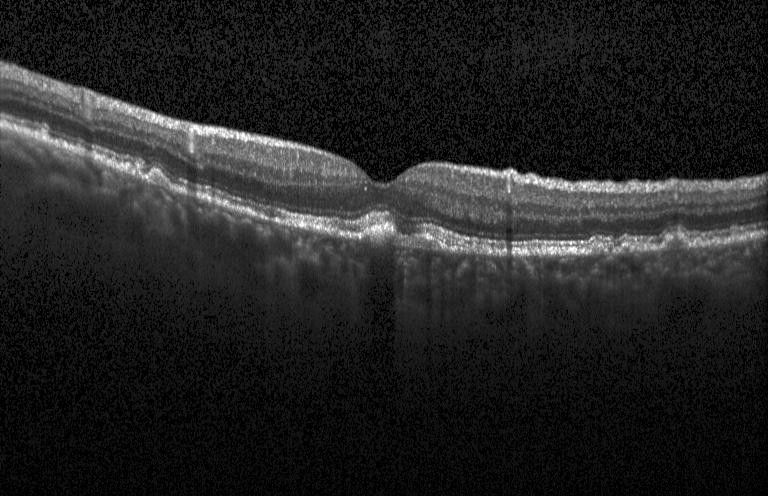

The scan shows sub-RPE drusenoid deposits.